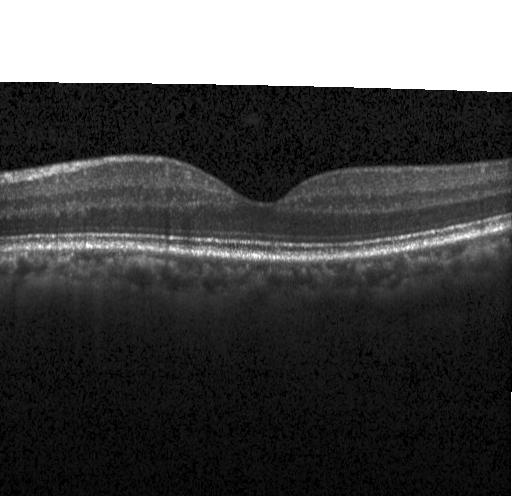 Retinal OCT cross-section showing no CNV, DME, or drusen.